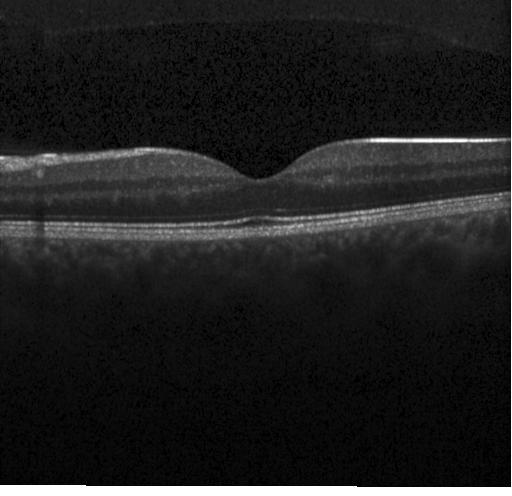

Spectral-domain OCT · instrument: Heidelberg Spectralis · centered on the fovea · optical coherence tomography scan.
Diagnosis: no evidence of CNV, DME, or drusen.